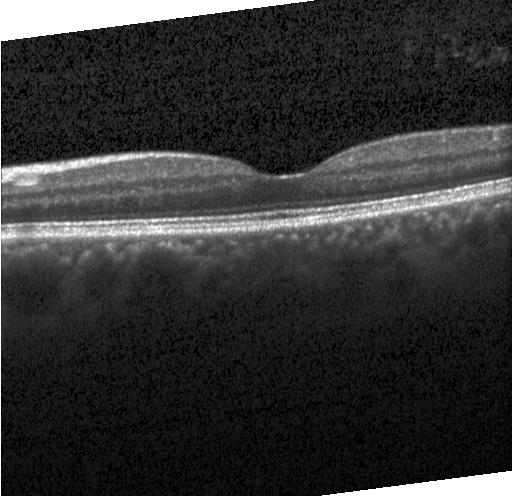
Optical coherence tomography scan. This B-scan demonstrates no evidence of choroidal neovascularization, diabetic macular edema, or drusen.